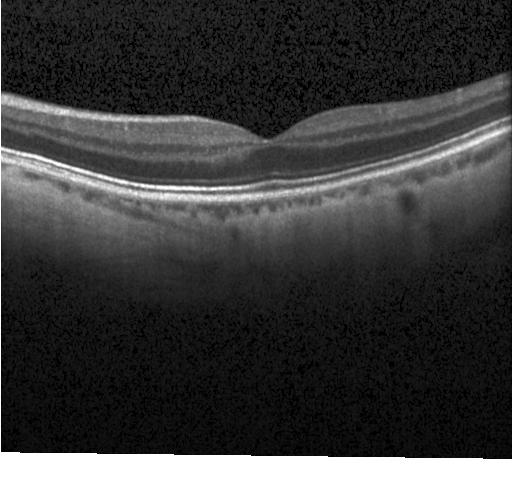
Retinal OCT cross-section · spectral-domain optical coherence tomography. Finding: no CNV, DME, or drusen.